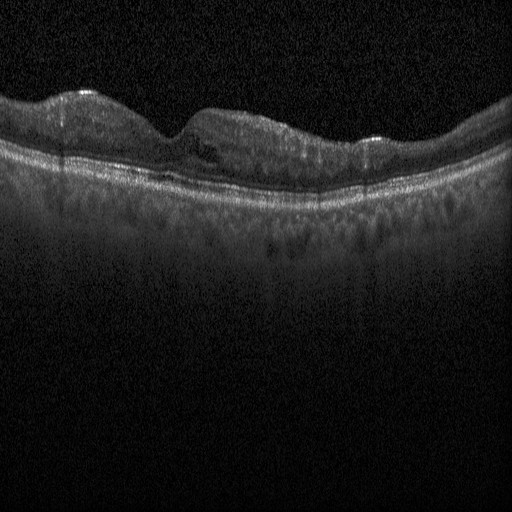

OCT finding: diabetic macular edema (DME).